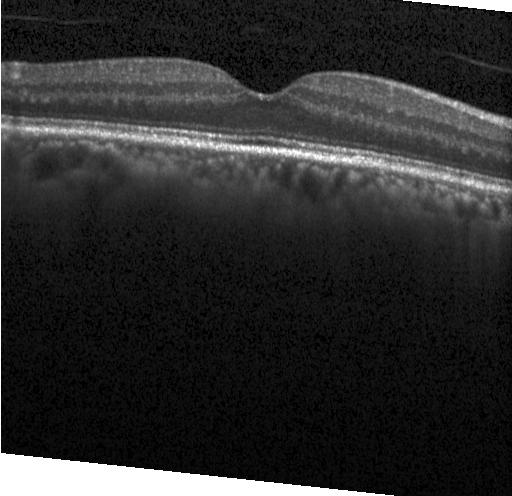

Fovea-centered · SD-OCT · OCT B-scan · Heidelberg Spectralis. Diagnosis: neither CNV, DME, nor drusen.